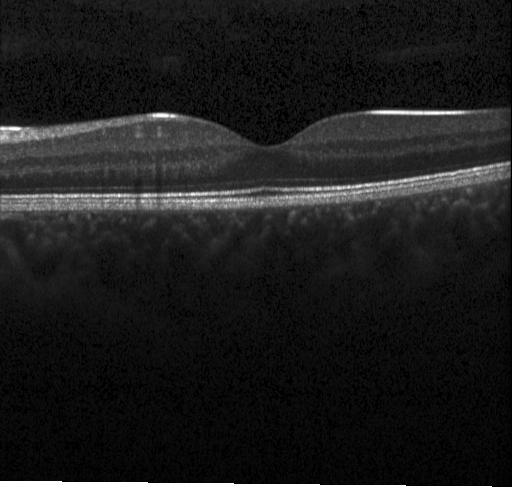
Macular OCT: neither choroidal neovascularization, diabetic macular edema, nor drusen.